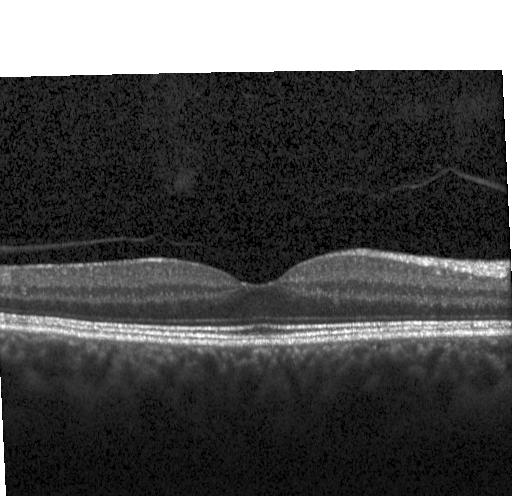 Dx: no CNV, DME, or drusen.